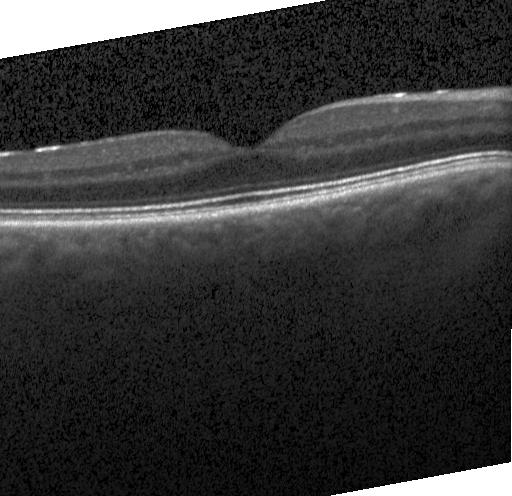
OCT line scan · spectral-domain optical coherence tomography · through the macula · Heidelberg Spectralis.
Neither choroidal neovascularization, diabetic macular edema, nor drusen.